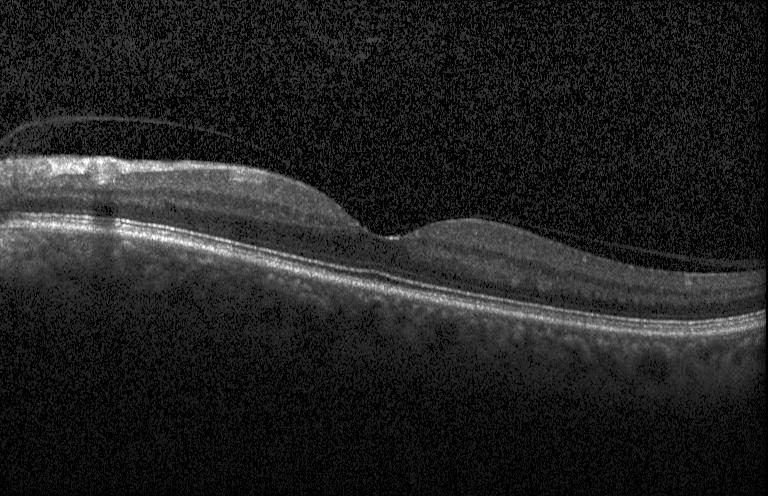
Through the macula; Heidelberg Spectralis; spectral-domain optical coherence tomography; retinal OCT B-scan. Impression: no evidence of choroidal neovascularization, diabetic macular edema, or drusen.